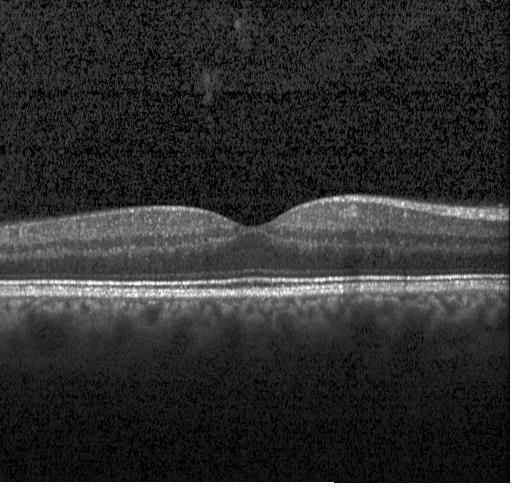
Neither choroidal neovascularization, diabetic macular edema, nor drusen.